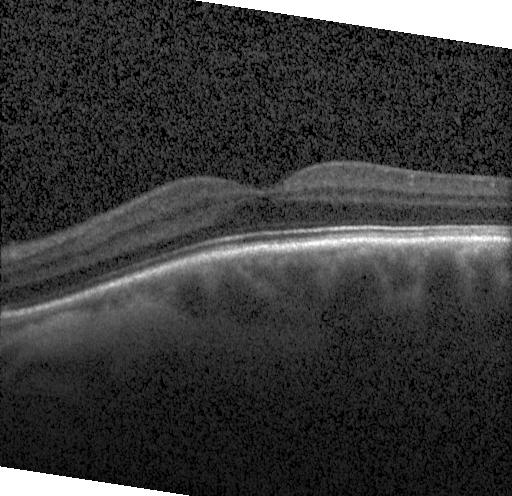 OCT finding: no evidence of CNV, DME, or drusen.